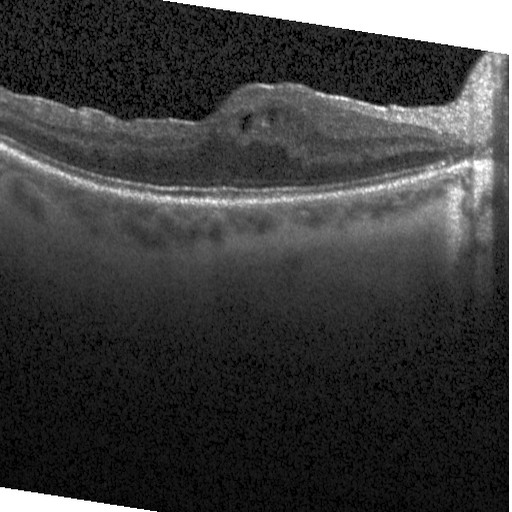
Spectral-domain OCT, optical coherence tomography scan. Impression: diabetic macular edema (DME).